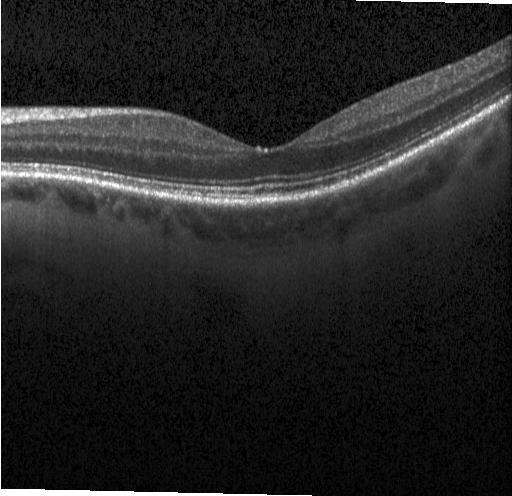

Spectral-domain optical coherence tomography · acquired on a Heidelberg Spectralis · OCT B-scan · fovea-centered — OCT finding: neither CNV, DME, nor drusen.